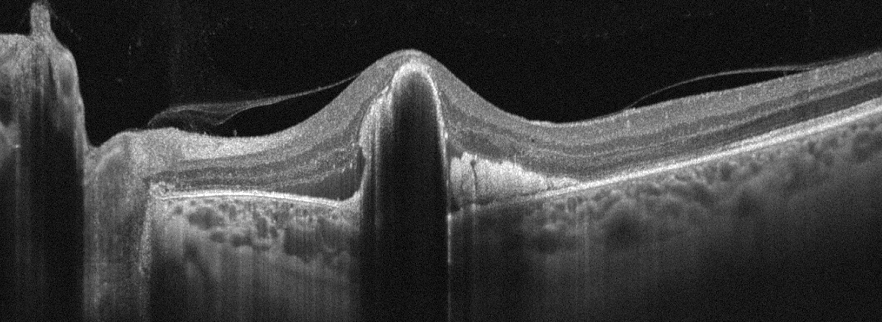 Retinal OCT B-scan; oculus sinister.
Age-related macular degeneration (AMD).